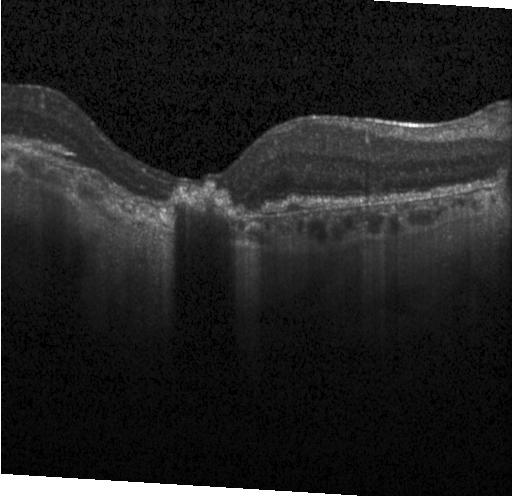

Fovea-centered. Optical coherence tomography B-scan. Spectral-domain OCT. Heidelberg Spectralis OCT system
Diagnosis: a choroidal neovascular membrane.